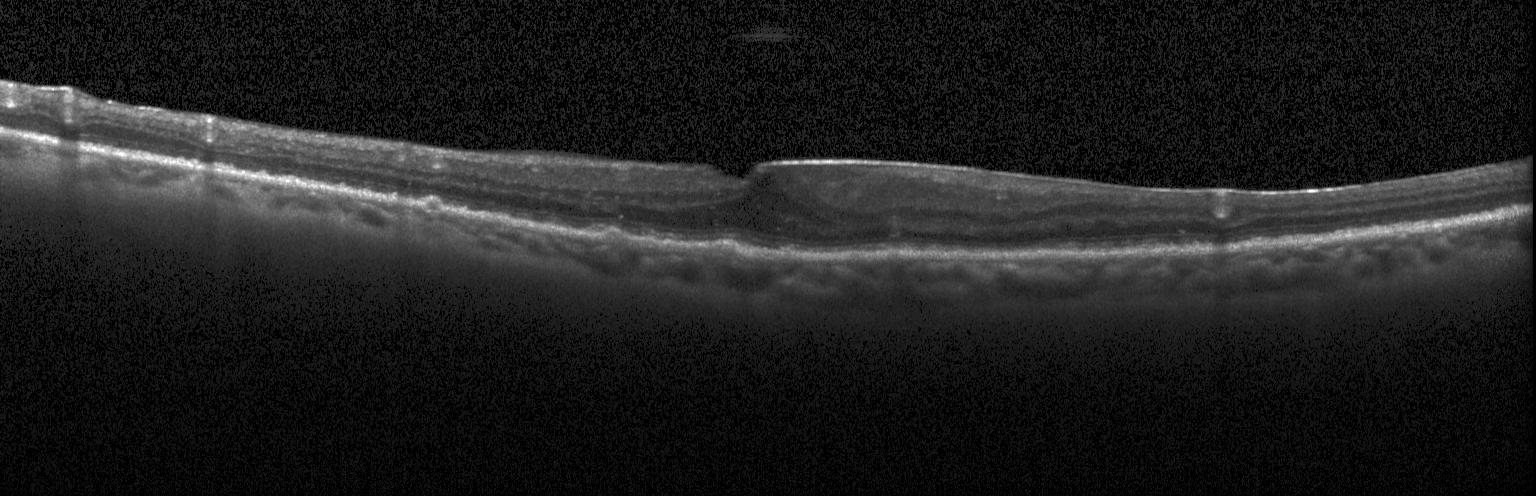 OCT line scan.
The scan shows multiple drusen.